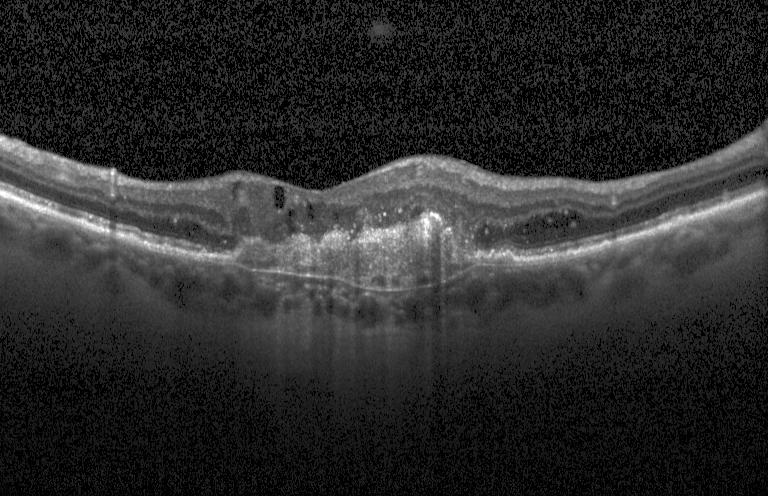

Retinal OCT cross-section. Diagnosis: choroidal neovascularization (CNV).